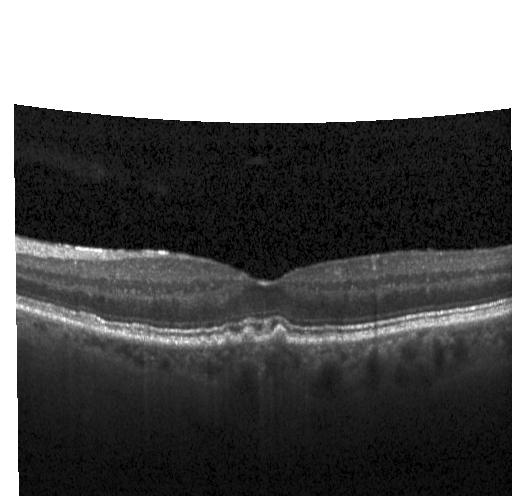 OCT line scan, SD-OCT, instrument: Heidelberg Spectralis
This B-scan demonstrates multiple drusen.